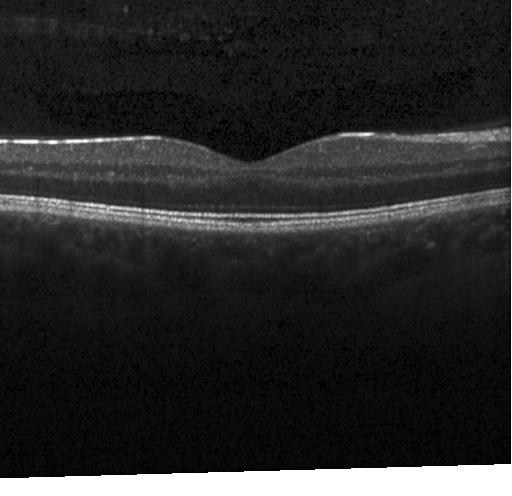

Macular OCT: no evidence of choroidal neovascularization, diabetic macular edema, or drusen.